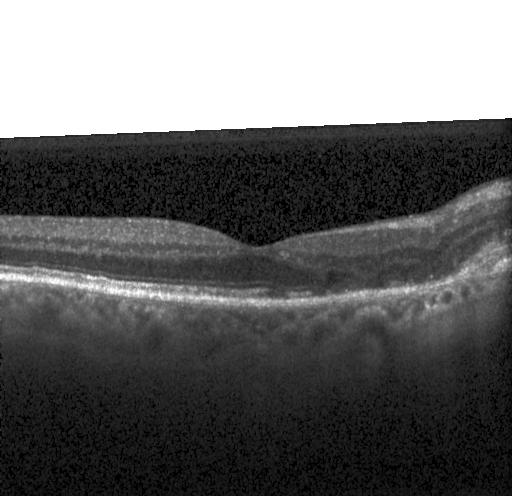

CNV.